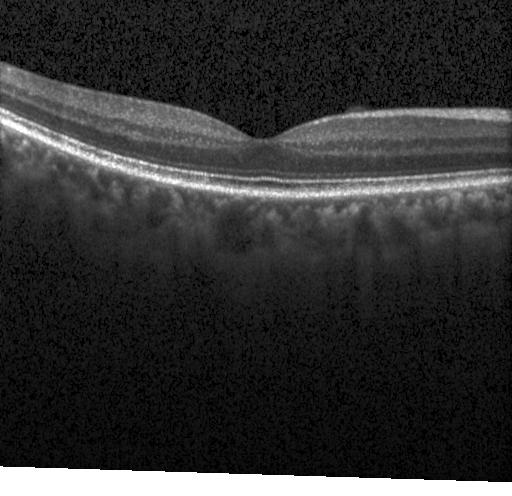
OCT B-scan showing no choroidal neovascularization, no diabetic macular edema, and no drusen.